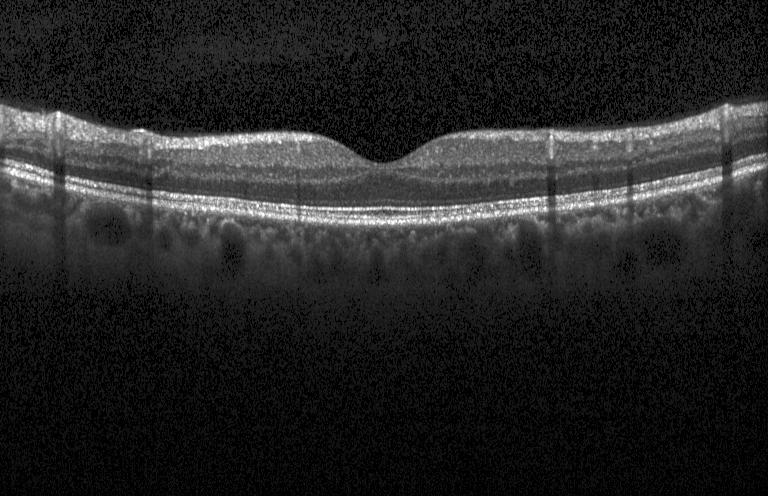

Spectral-domain OCT B-scan: neither choroidal neovascularization, diabetic macular edema, nor drusen.